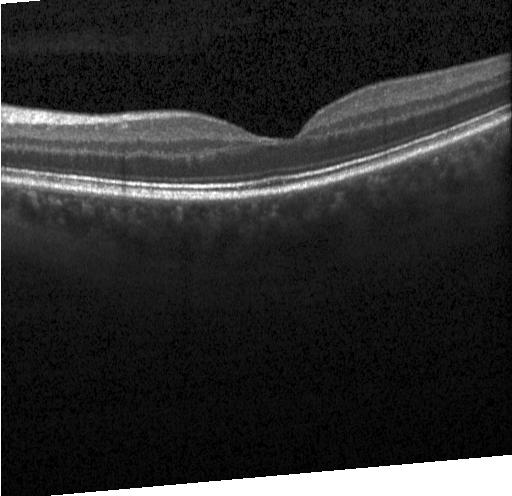

OCT line scan.
Macular OCT: no CNV, no DME, and no drusen.